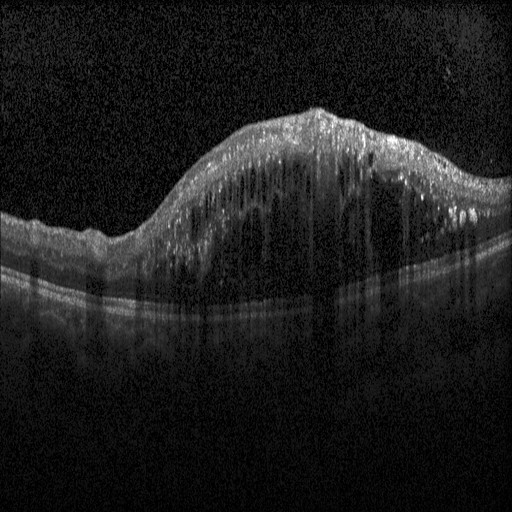 Macular OCT: diabetic macular edema (DME).